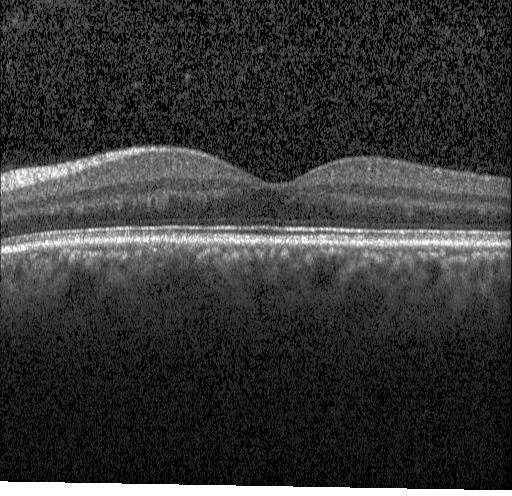 Retinal OCT B-scan, spectral-domain optical coherence tomography. Impression: no choroidal neovascularization, no diabetic macular edema, and no drusen.